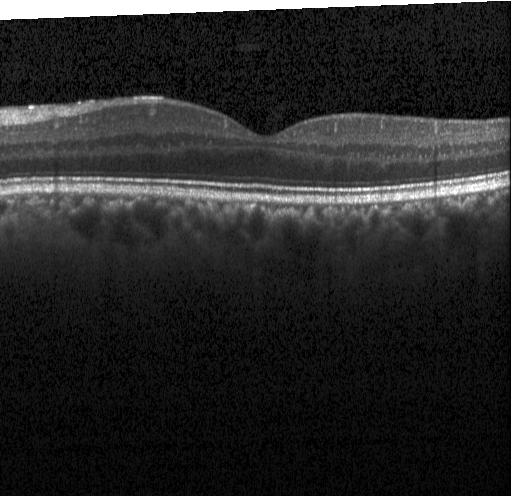
Horizontal scan through the fovea, retinal OCT cross-section
Impression: no evidence of choroidal neovascularization, diabetic macular edema, or drusen.